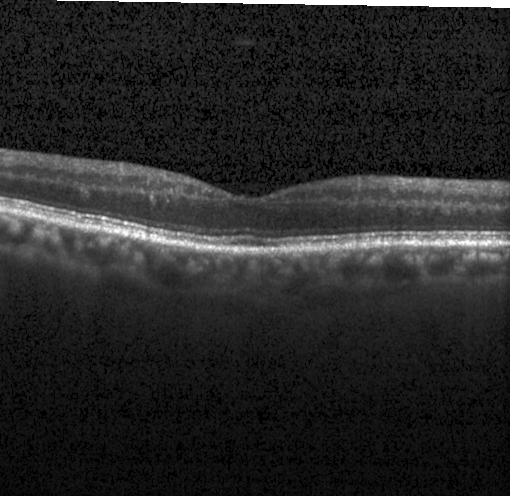
Through the macula, Heidelberg Spectralis, retinal OCT B-scan, spectral-domain OCT. Finding: no choroidal neovascularization, diabetic macular edema, or drusen.